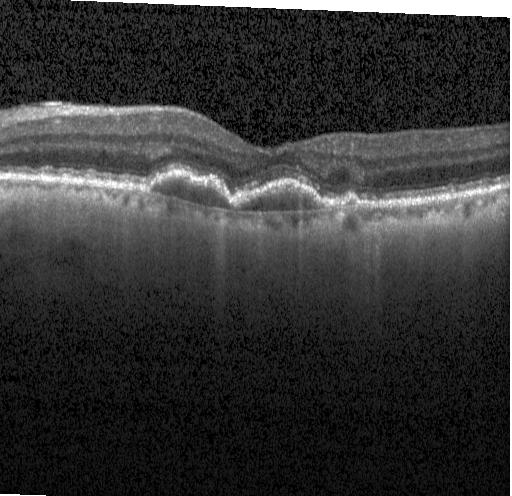

Macular scan · Heidelberg Spectralis OCT system · OCT B-scan · spectral-domain optical coherence tomography
Impression: a choroidal neovascular membrane.